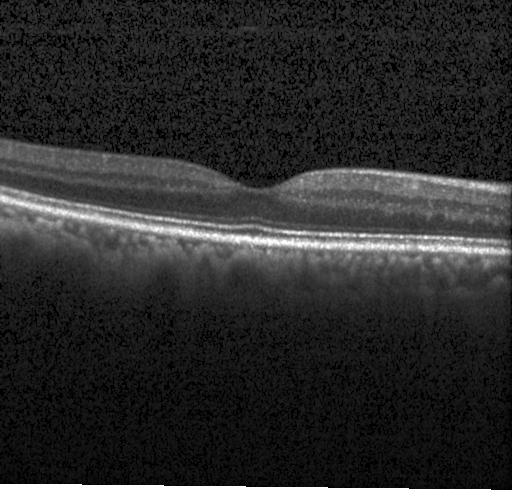

Spectral-domain optical coherence tomography · acquired on a Heidelberg Spectralis · optical coherence tomography scan. Finding: no CNV, no DME, and no drusen.